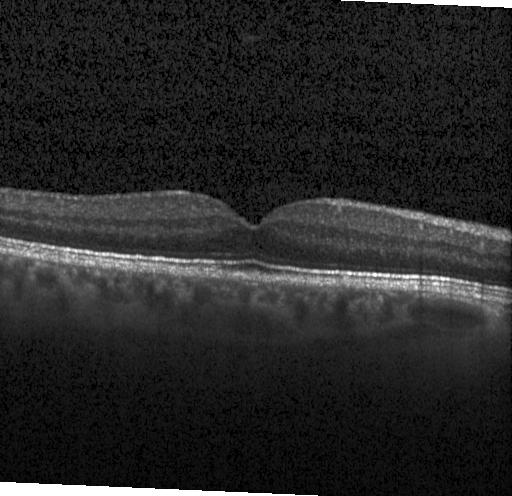

Optical coherence tomography B-scan; macular scan. No CNV, DME, or drusen.